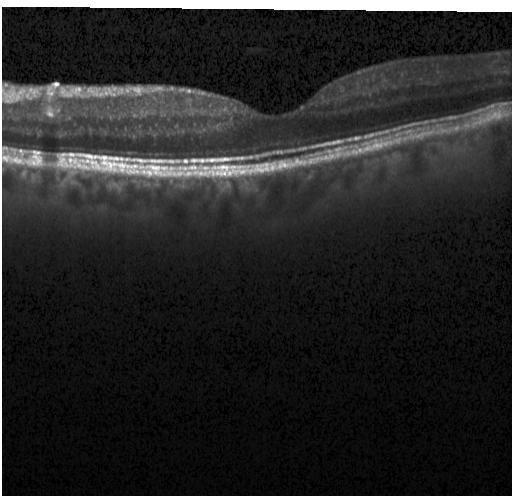

Diagnosis: neither choroidal neovascularization, diabetic macular edema, nor drusen.